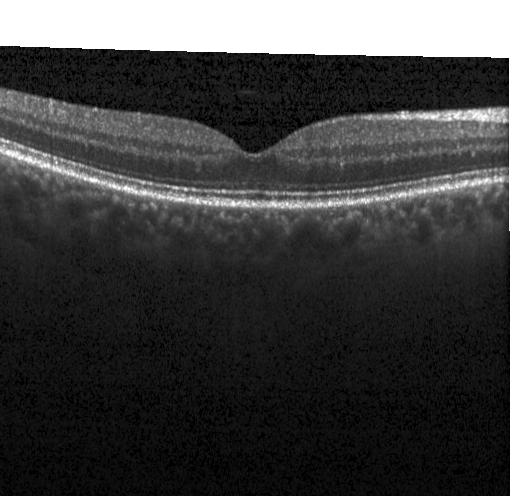

Spectral-domain optical coherence tomography. Centered on the fovea. OCT line scan. Heidelberg Spectralis.
Finding: neither choroidal neovascularization, diabetic macular edema, nor drusen.